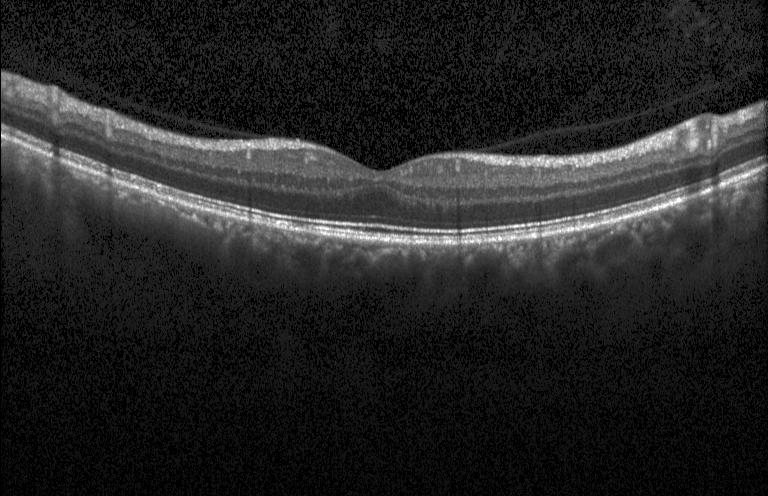 Impression: no choroidal neovascularization, no diabetic macular edema, and no drusen.